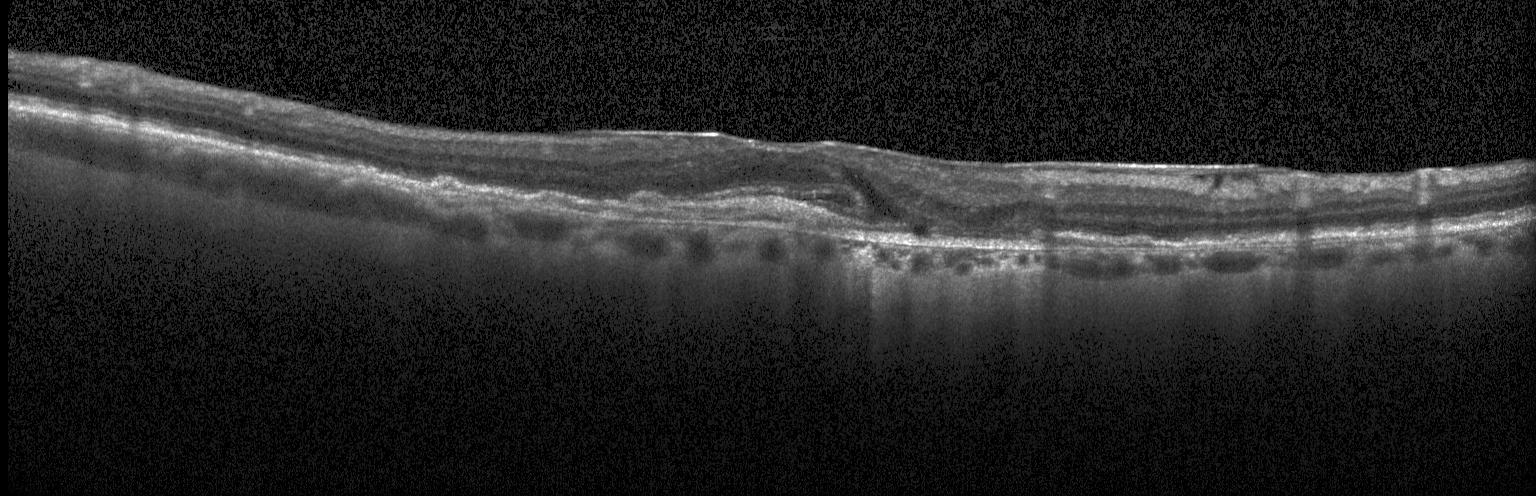

Spectral-domain OCT, fovea-centered, retinal OCT cross-section, instrument: Heidelberg Spectralis. This B-scan demonstrates CNV.